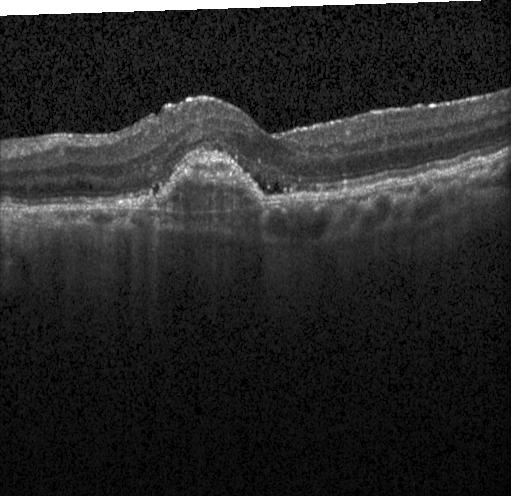 Retinal OCT cross-section · through the macula
A choroidal neovascular membrane.